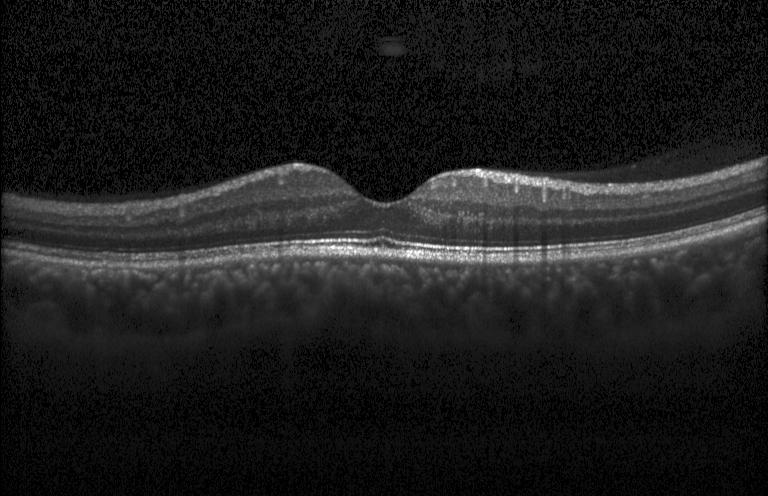

Spectral-domain optical coherence tomography · Heidelberg Spectralis OCT system · through the macula · optical coherence tomography scan. Dx: no choroidal neovascularization, diabetic macular edema, or drusen.